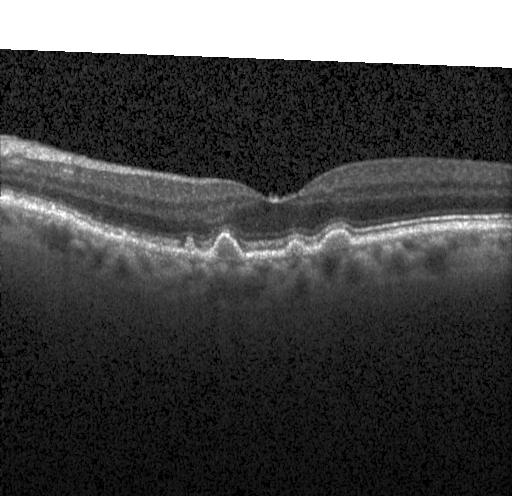 Retinal OCT cross-section — Impression: drusen.